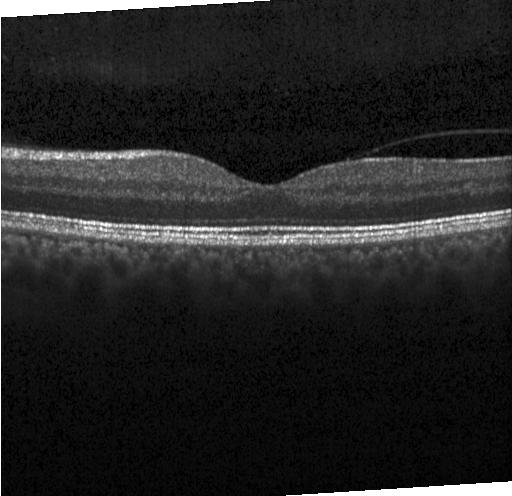

Retinal OCT cross-section, centered on the fovea
This B-scan demonstrates no CNV, no DME, and no drusen.